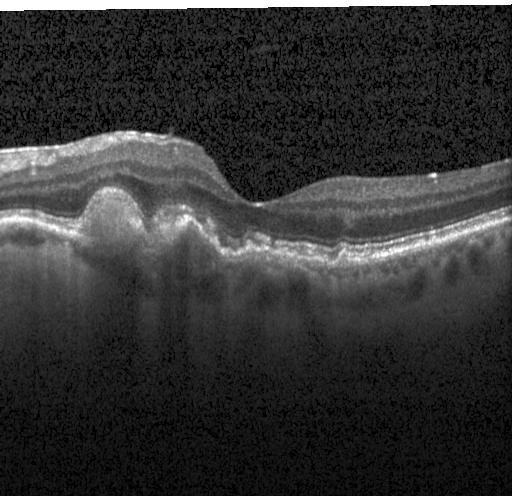

Heidelberg Spectralis OCT system · retinal OCT cross-section.
Impression: a choroidal neovascular membrane.